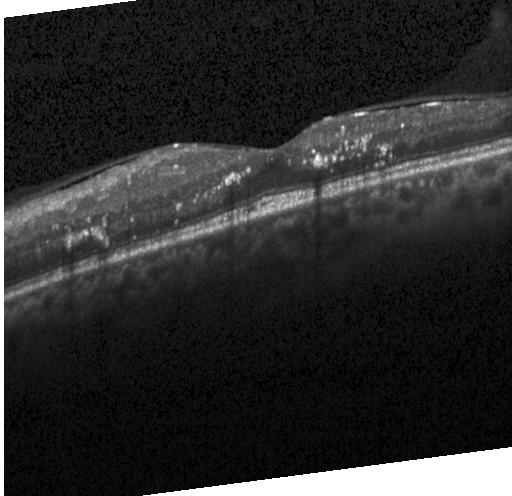
Spectral-domain optical coherence tomography. Macular scan. OCT B-scan.
Dx: DME.